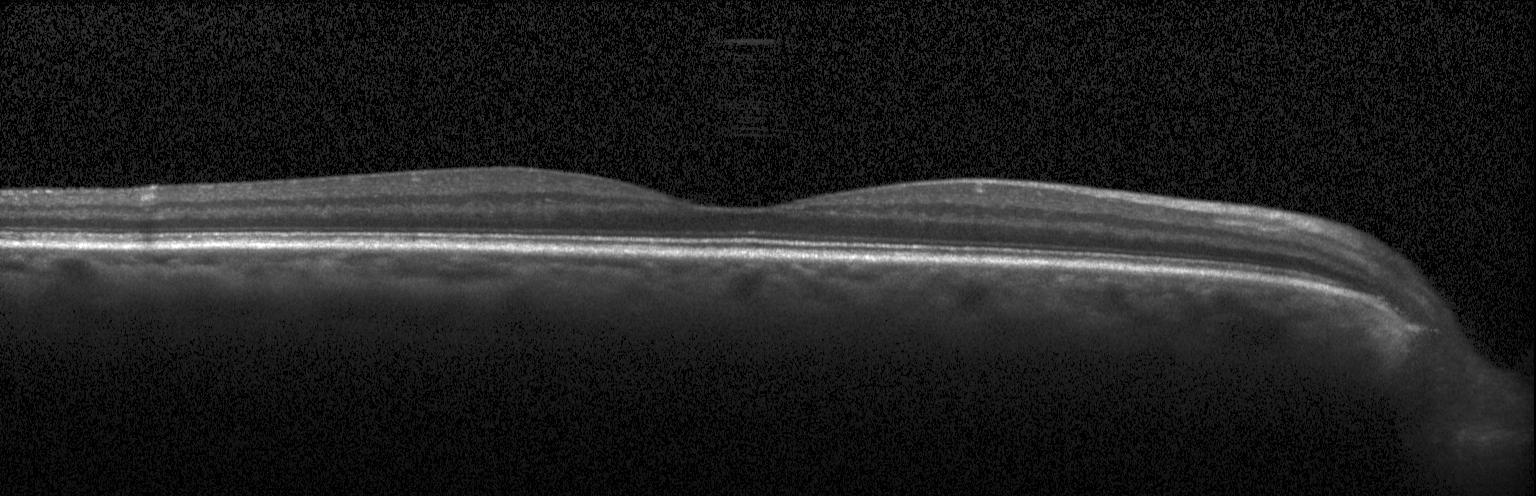

Retinal OCT cross-section. Instrument: Heidelberg Spectralis. SD-OCT — No evidence of CNV, DME, or drusen.